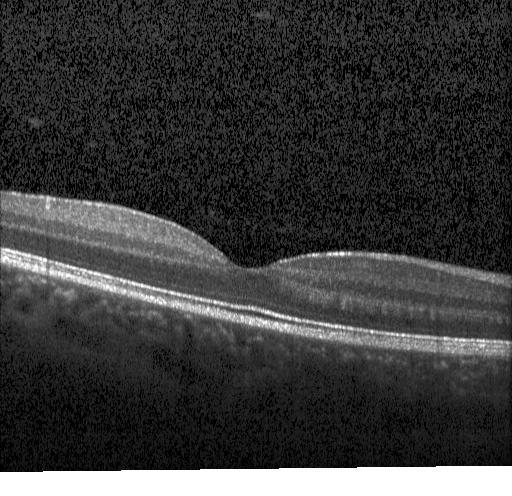
Heidelberg Spectralis OCT system. OCT line scan. Spectral-domain OCT. Fovea-centered. This B-scan demonstrates neither choroidal neovascularization, diabetic macular edema, nor drusen.